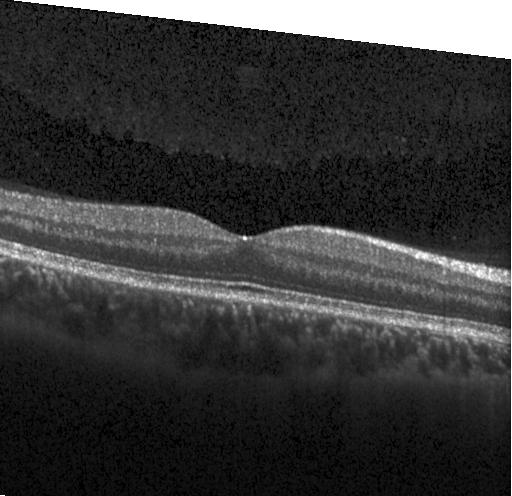

Horizontal scan through the fovea. OCT B-scan. The scan shows neither choroidal neovascularization, diabetic macular edema, nor drusen.